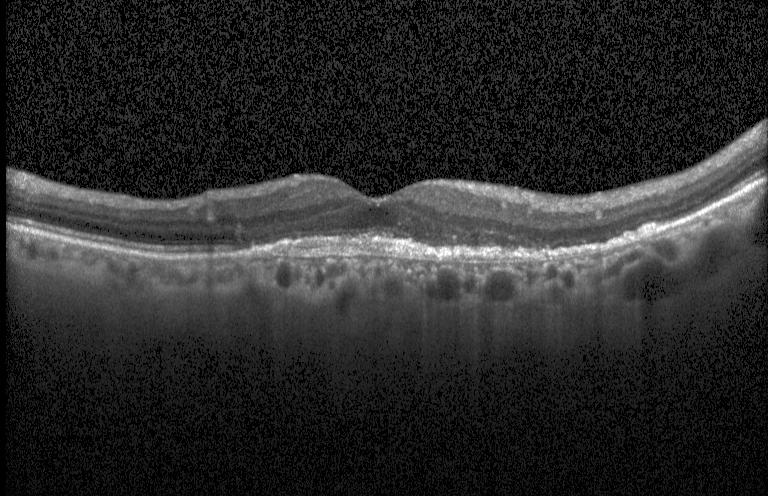 Instrument: Heidelberg Spectralis; retinal OCT cross-section — Impression: choroidal neovascularization.